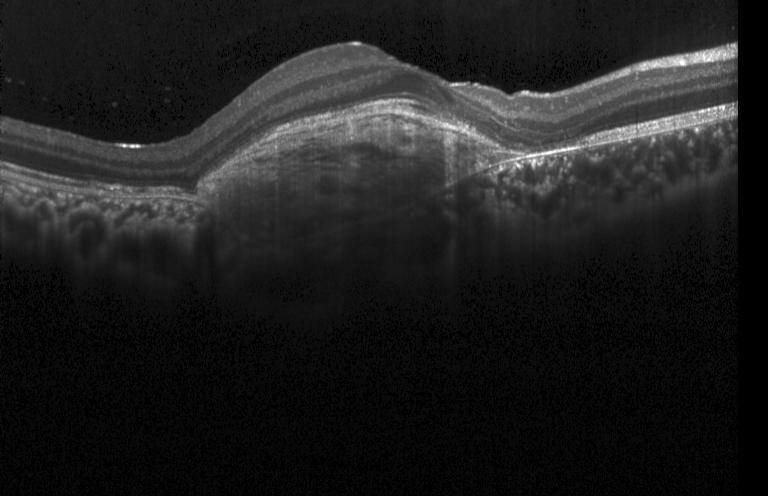 A choroidal neovascular membrane.